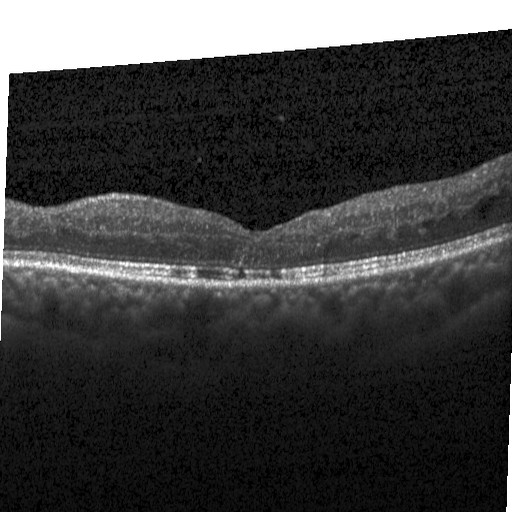 Impression: DME.